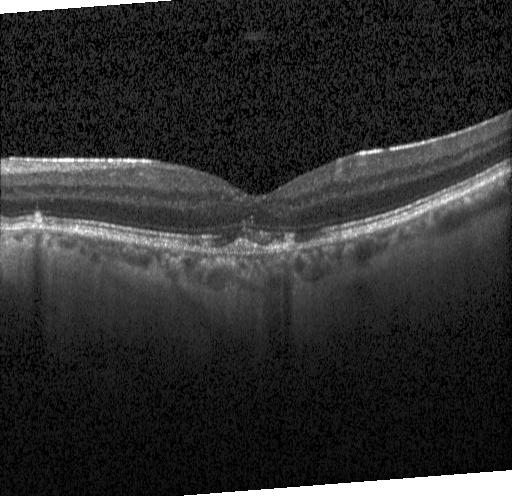

Retinal OCT cross-section — The scan shows choroidal neovascularization.